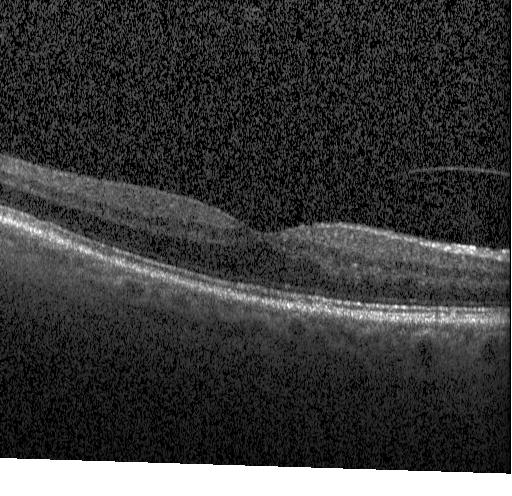 OCT B-scan showing neither CNV, DME, nor drusen.